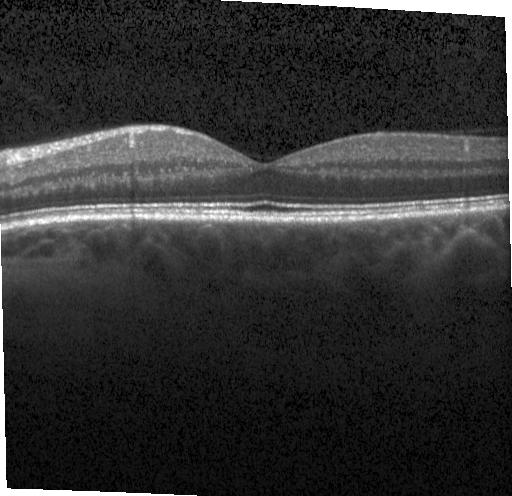
Retinal OCT B-scan, Heidelberg Spectralis — Impression: neither choroidal neovascularization, diabetic macular edema, nor drusen.